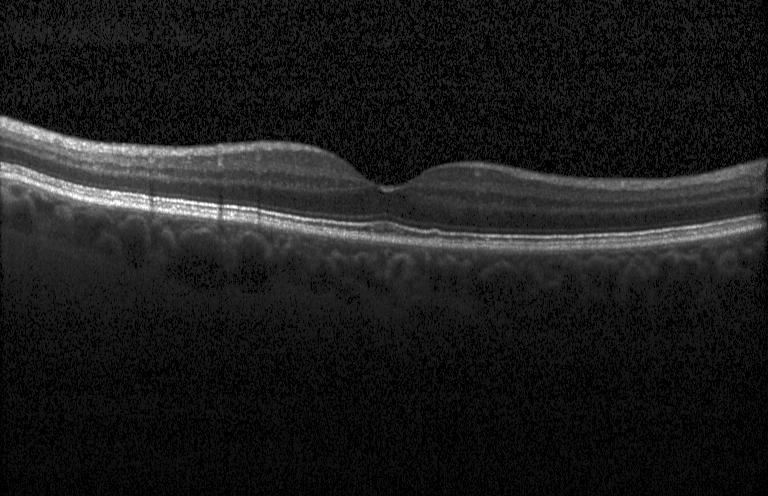
Macular scan; OCT line scan; spectral-domain optical coherence tomography
Assessment: no evidence of choroidal neovascularization, diabetic macular edema, or drusen.